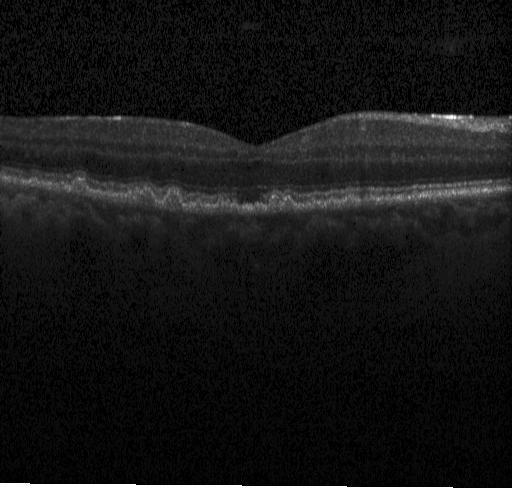

Diagnosis: multiple drusen.